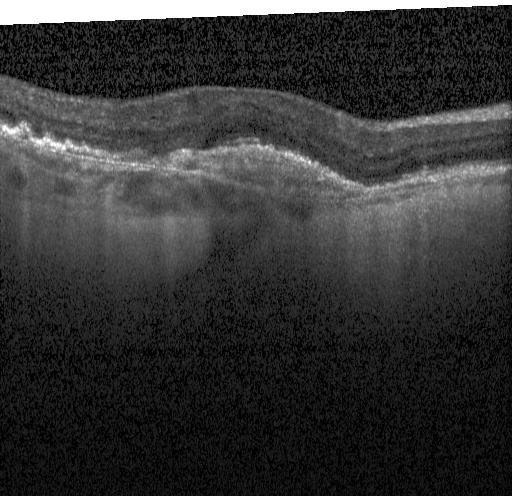
Retinal OCT cross-section, horizontal scan through the fovea, SD-OCT
Diagnosis: choroidal neovascularization (CNV).